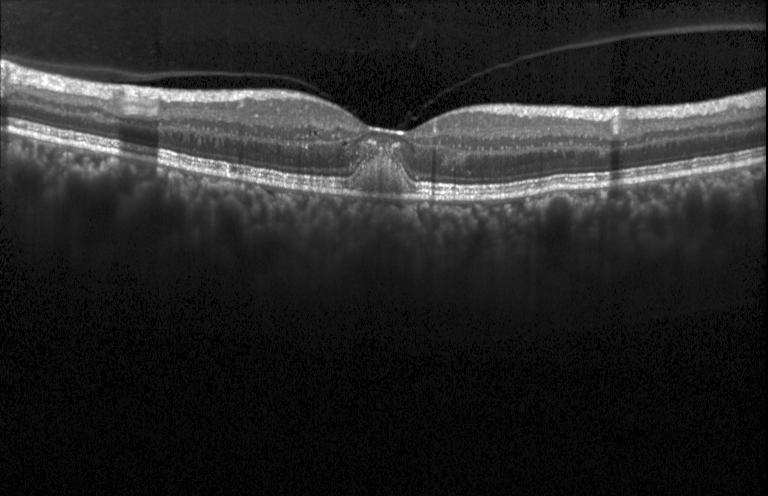 Heidelberg Spectralis; optical coherence tomography B-scan.
Dx: choroidal neovascularization.